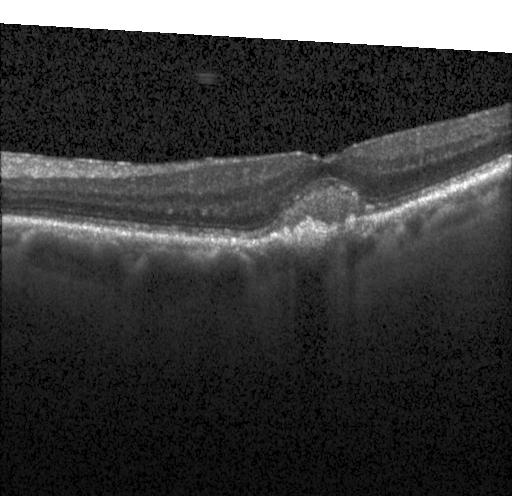 SD-OCT, optical coherence tomography B-scan
The scan shows choroidal neovascularization (CNV).